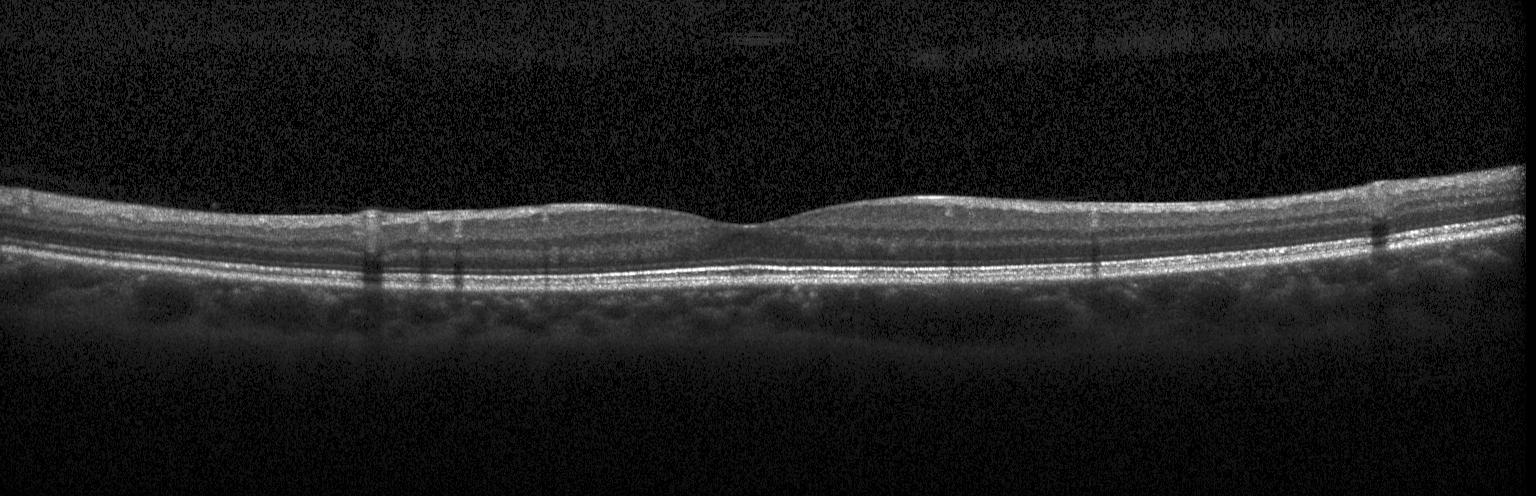

Finding: neither CNV, DME, nor drusen.